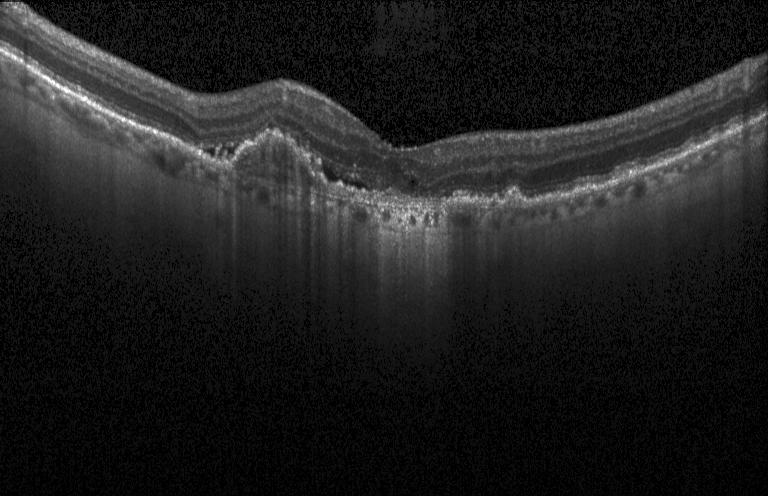 Spectral-domain OCT B-scan: a choroidal neovascular membrane.